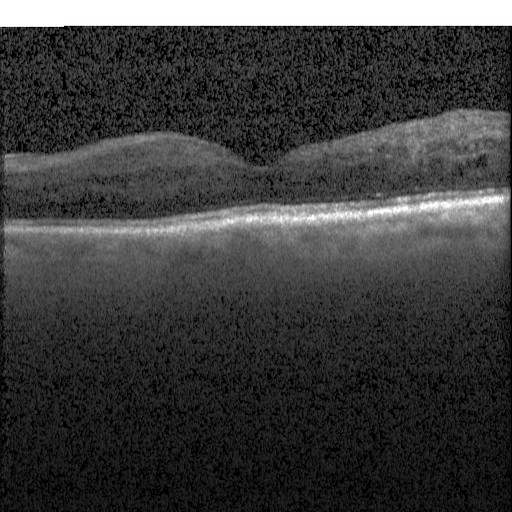

Optical coherence tomography B-scan
Macular OCT: diabetic macular edema (DME).